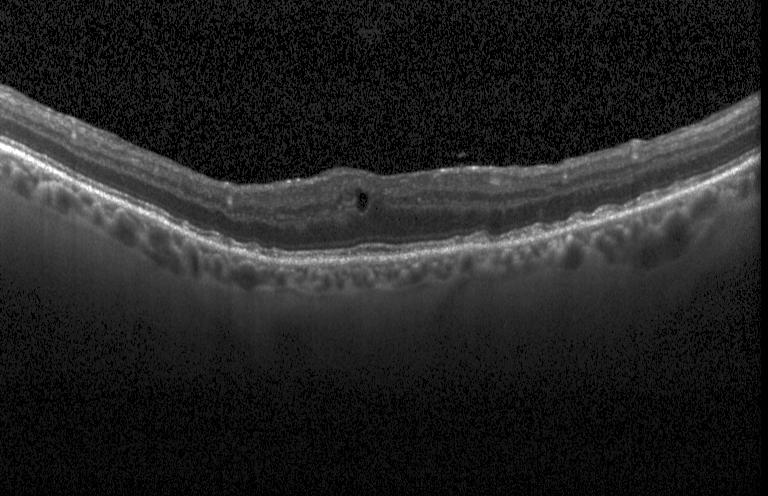

The scan shows diabetic macular edema.